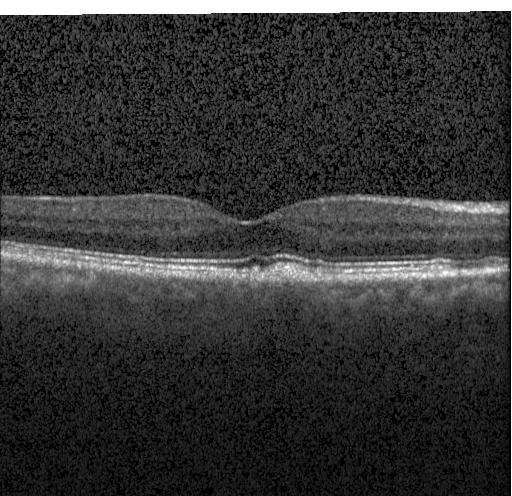

OCT B-scan, through the macula, acquired on a Heidelberg Spectralis.
Diagnosis: sub-RPE drusenoid deposits.